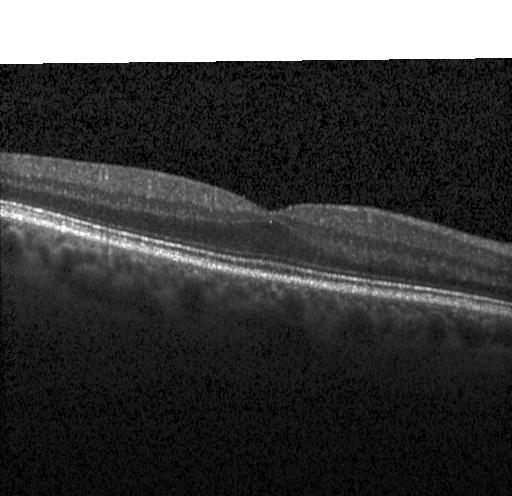
OCT scan showing no CNV, no DME, and no drusen.